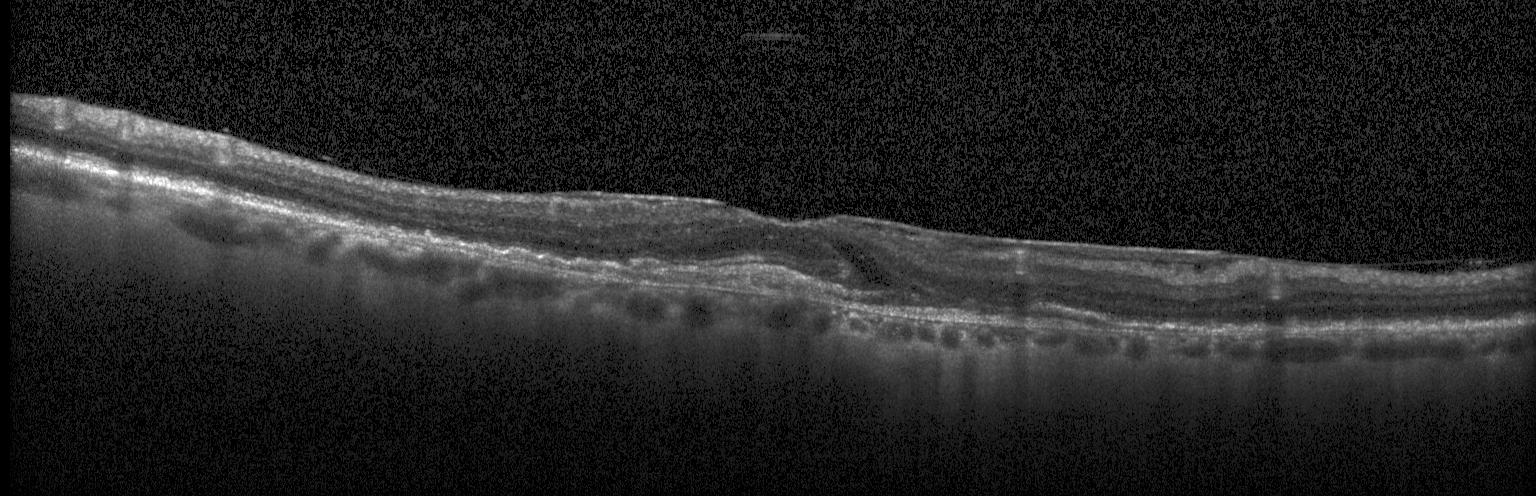 Macular OCT demonstrating a choroidal neovascular membrane.